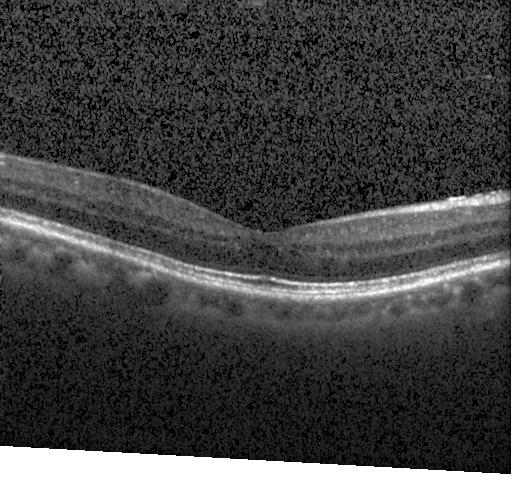 OCT B-scan
Finding: no evidence of choroidal neovascularization, diabetic macular edema, or drusen.